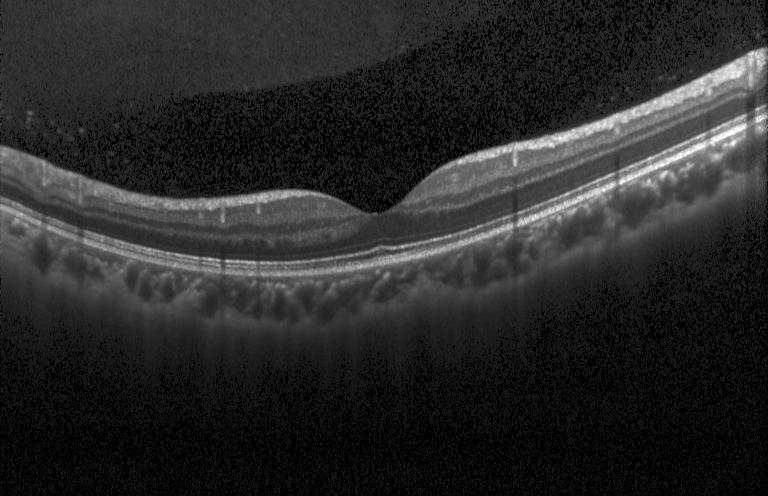 Spectral-domain optical coherence tomography; retinal OCT B-scan.
Finding: no evidence of CNV, DME, or drusen.